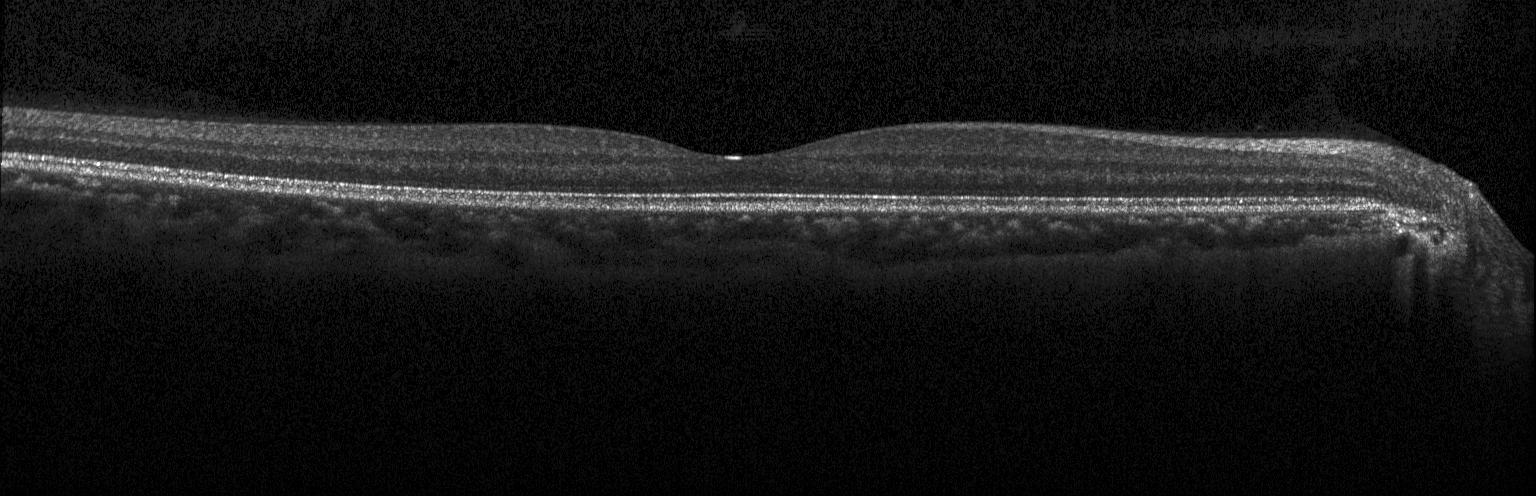
Through the macula; acquired on a Heidelberg Spectralis; spectral-domain OCT; retinal OCT B-scan
Macular OCT: neither CNV, DME, nor drusen.